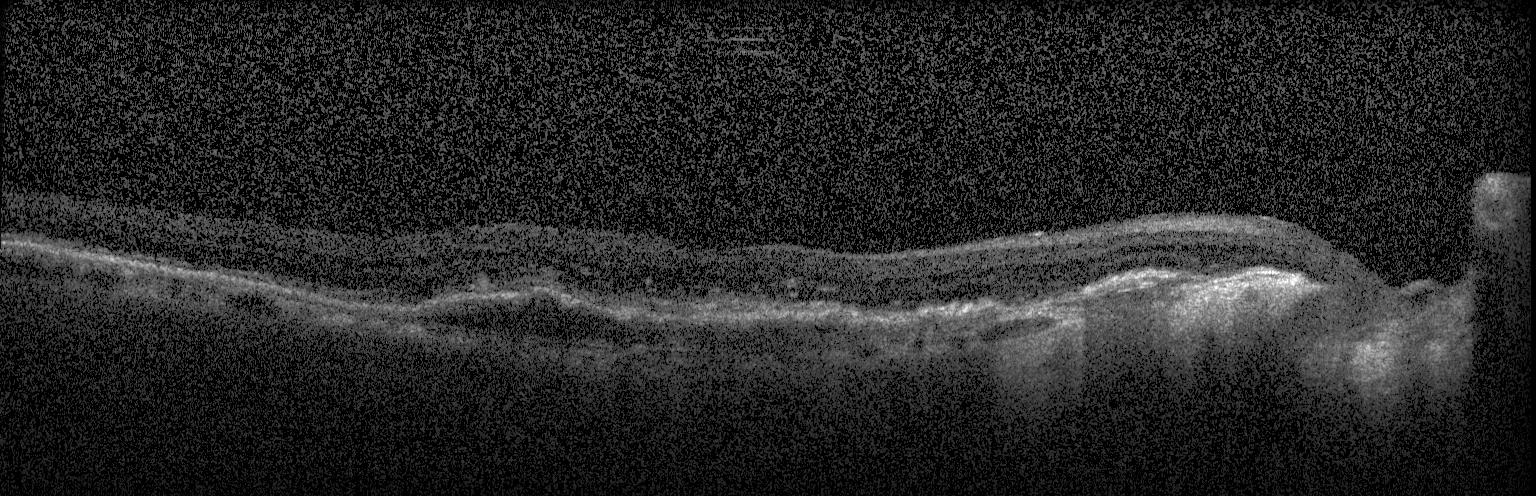
Diagnosis: a choroidal neovascular membrane.